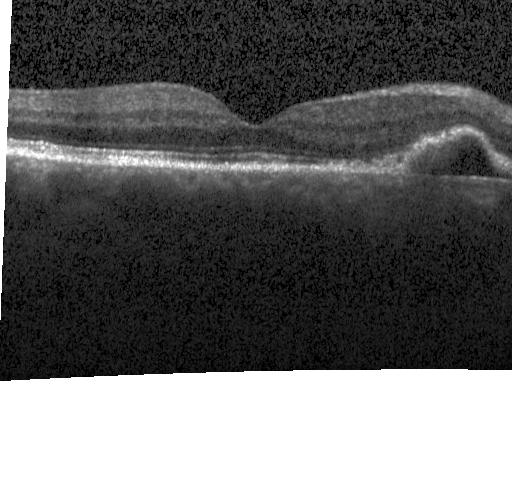
SD-OCT, retinal OCT B-scan.
Dx: CNV.